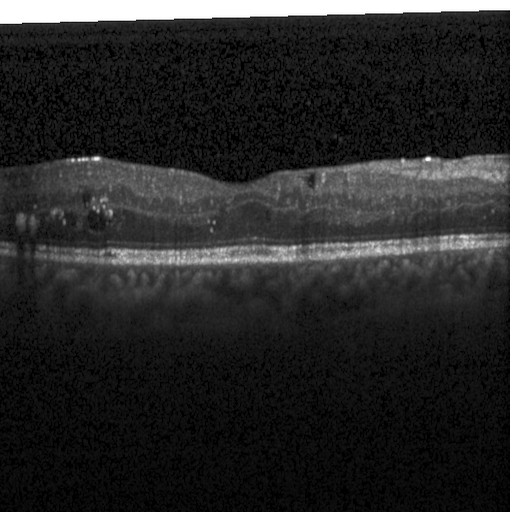 OCT B-scan.
OCT finding: DME.